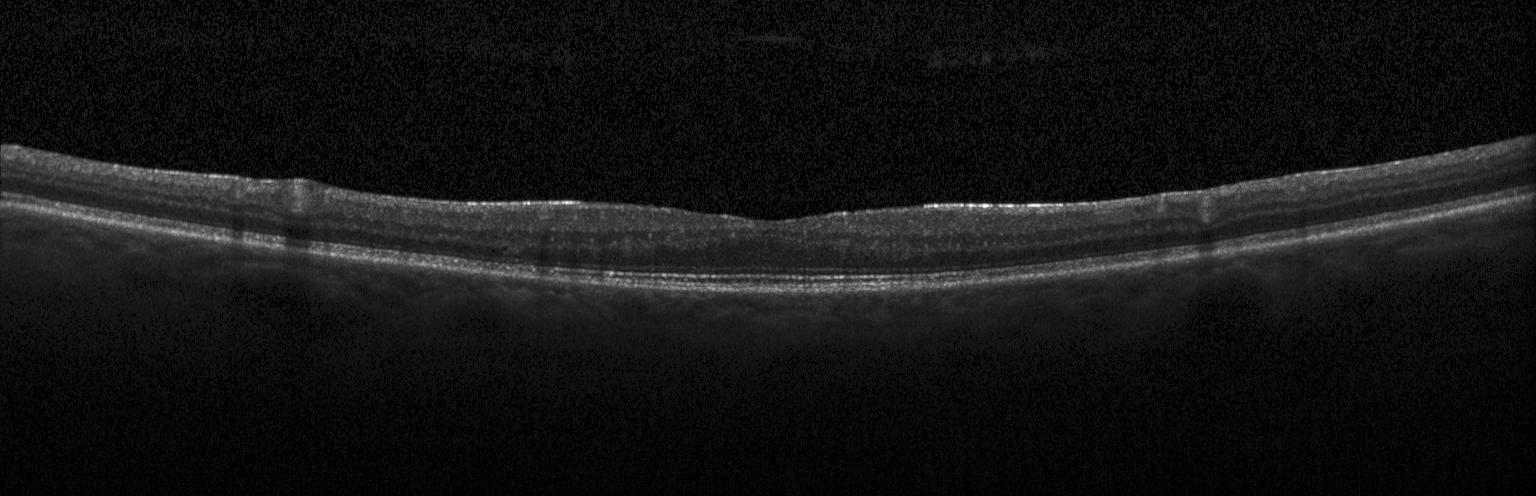

Fovea-centered. Spectral-domain OCT. Retinal OCT cross-section. Finding: no choroidal neovascularization, diabetic macular edema, or drusen.